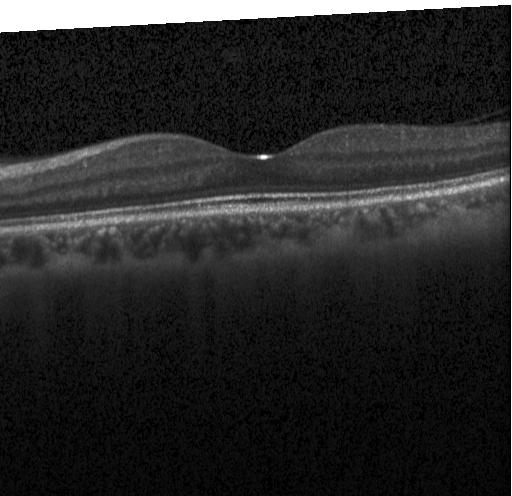 Retinal OCT cross-section showing no choroidal neovascularization, no diabetic macular edema, and no drusen.